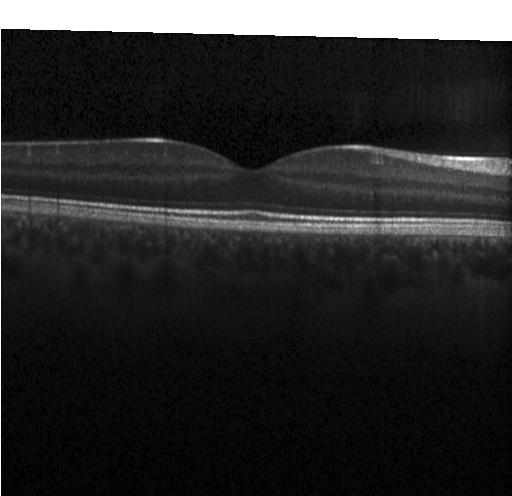
Spectral-domain OCT, fovea-centered, optical coherence tomography scan.
The scan shows no choroidal neovascularization, diabetic macular edema, or drusen.